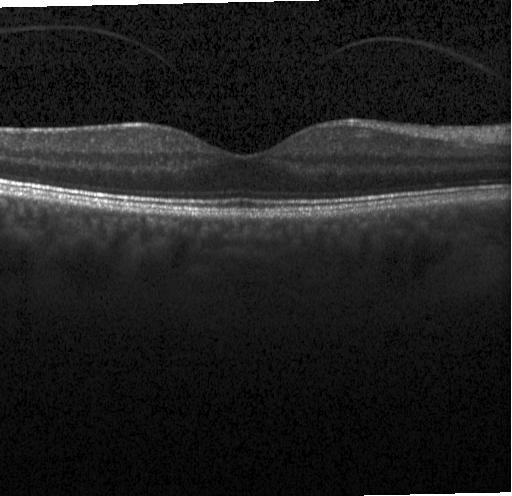

OCT finding: no CNV, no DME, and no drusen.